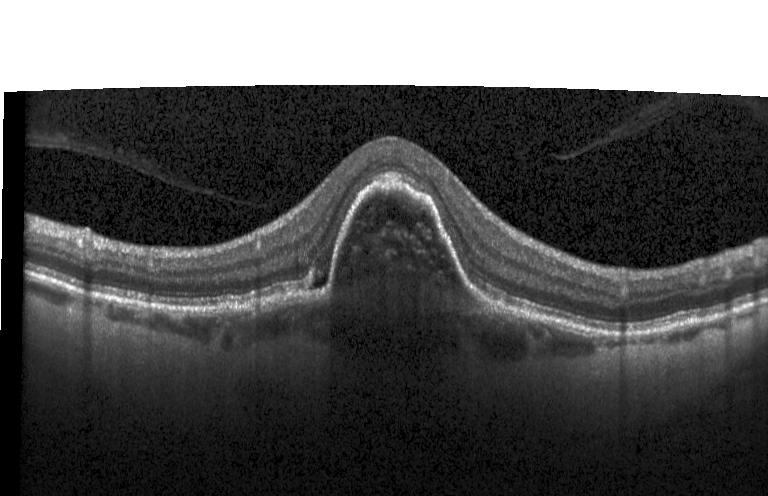

OCT finding: a choroidal neovascular membrane.